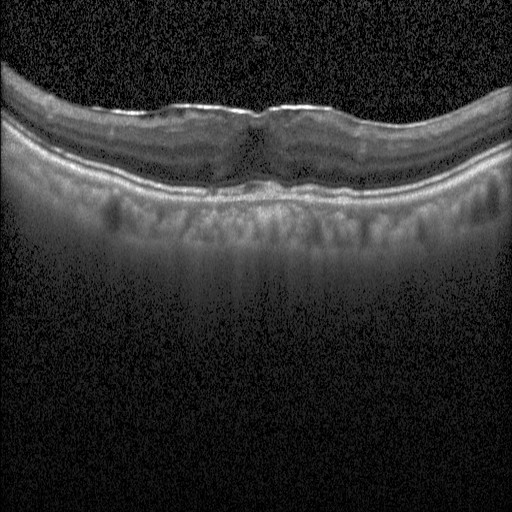

OCT line scan
Diabetic macular edema (DME).